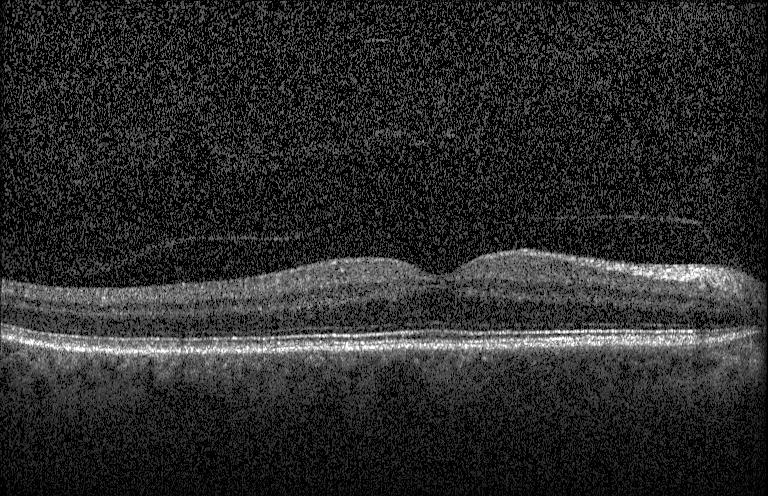

Spectral-domain optical coherence tomography. Optical coherence tomography scan.
This B-scan demonstrates no CNV, DME, or drusen.